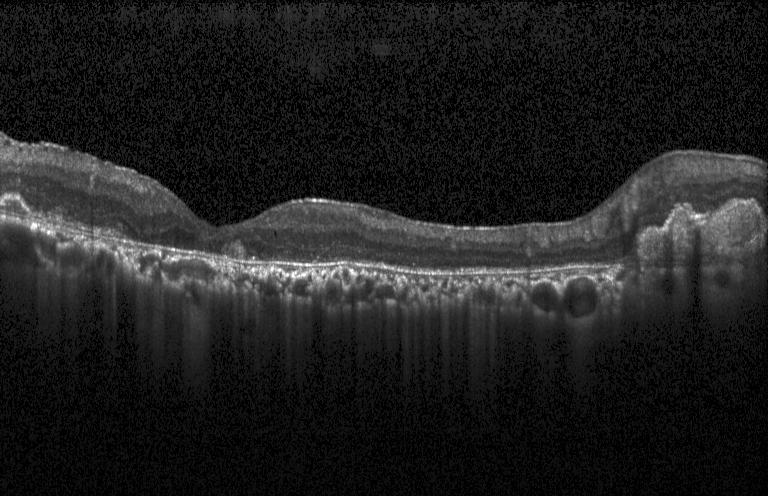

This B-scan demonstrates choroidal neovascularization (CNV).